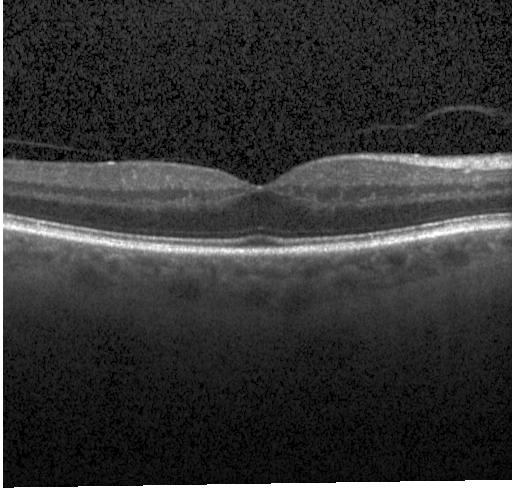

OCT B-scan showing neither choroidal neovascularization, diabetic macular edema, nor drusen.